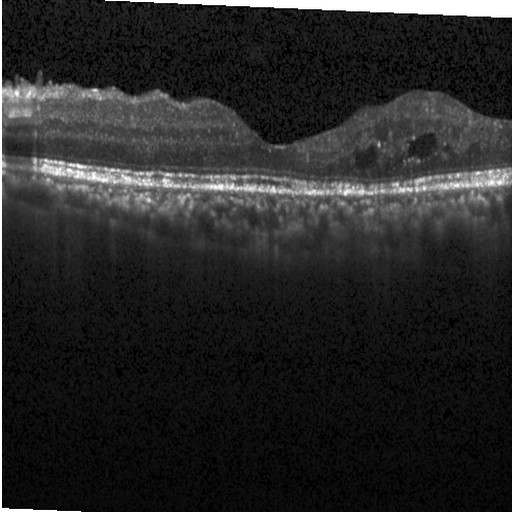 OCT B-scan, centered on the fovea — Diagnosis: diabetic macular edema.